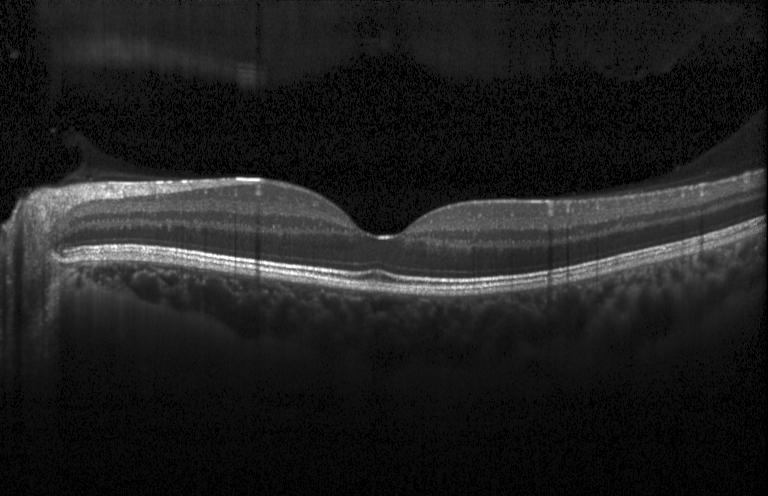

Diagnosis: neither choroidal neovascularization, diabetic macular edema, nor drusen.